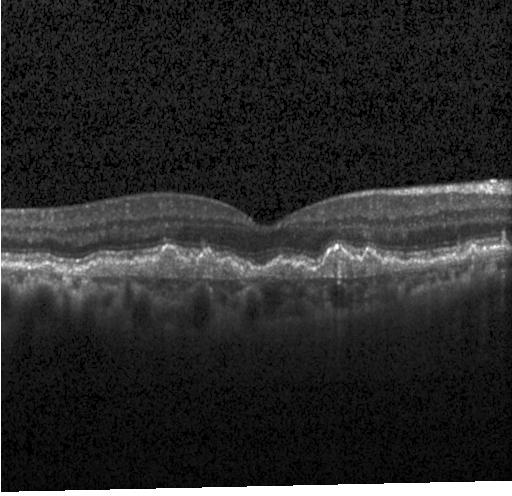 OCT finding: CNV.